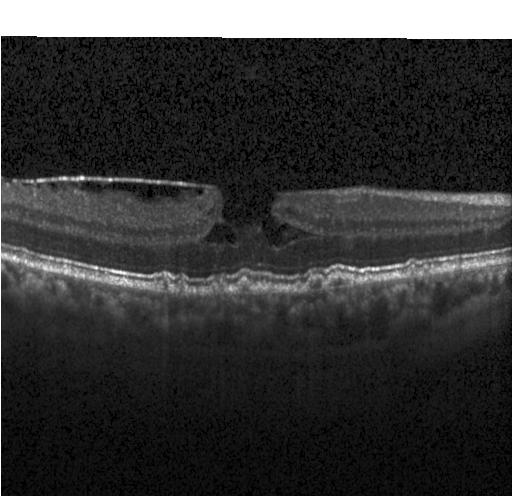

OCT line scan. Diagnosis: multiple drusen.